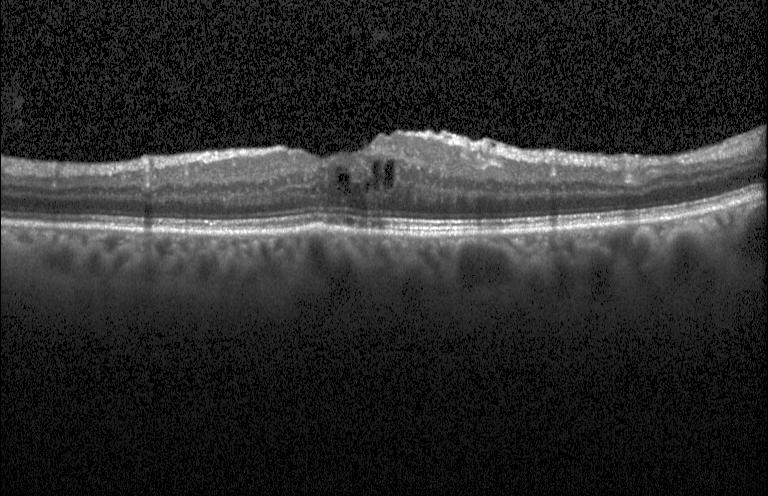 Finding: diabetic macular edema (DME).